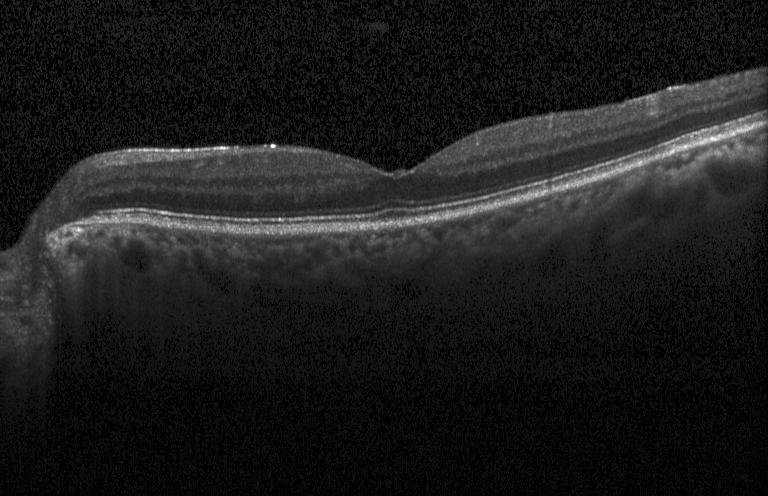

Spectral-domain OCT. Optical coherence tomography scan
Impression: no CNV, no DME, and no drusen.